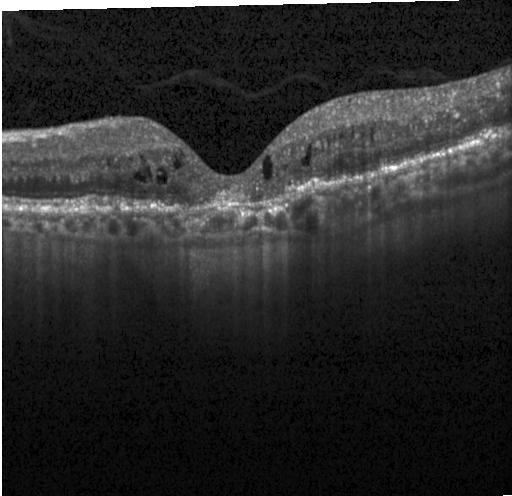
Finding: a choroidal neovascular membrane.